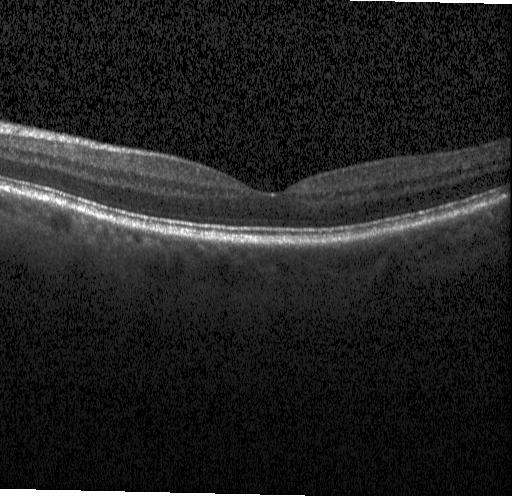 Through the macula · retinal OCT cross-section · spectral-domain OCT · acquired on a Heidelberg Spectralis
This B-scan demonstrates neither choroidal neovascularization, diabetic macular edema, nor drusen.